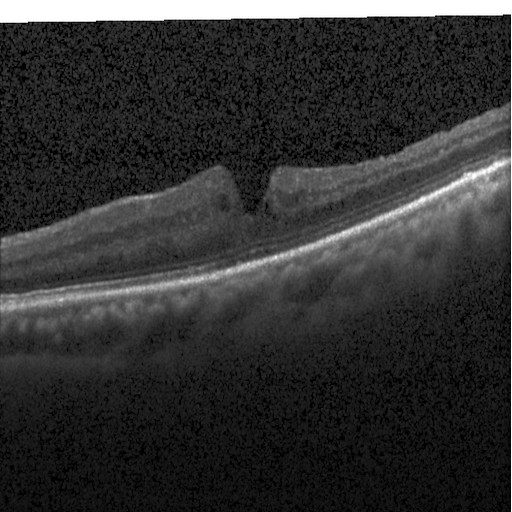 Diabetic macular edema.